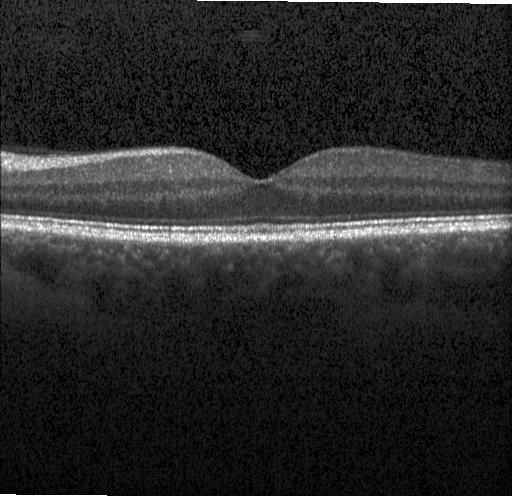
Optical coherence tomography scan. Macular scan. Impression: no evidence of choroidal neovascularization, diabetic macular edema, or drusen.